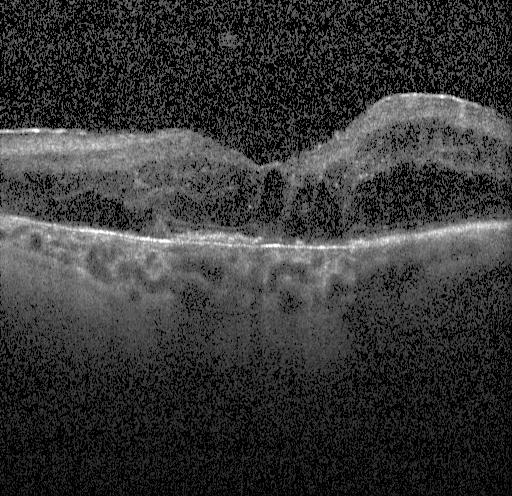
The scan shows CNV.